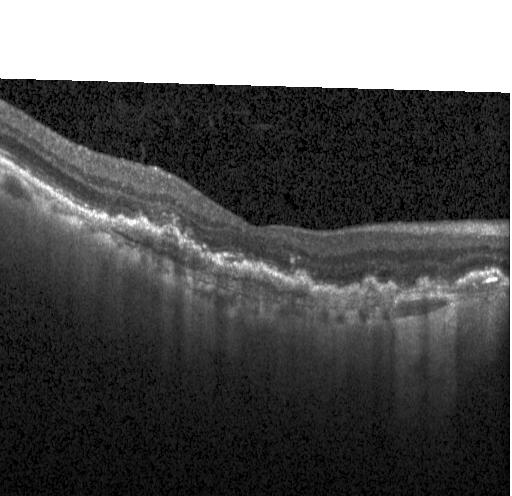 Impression: a choroidal neovascular membrane.